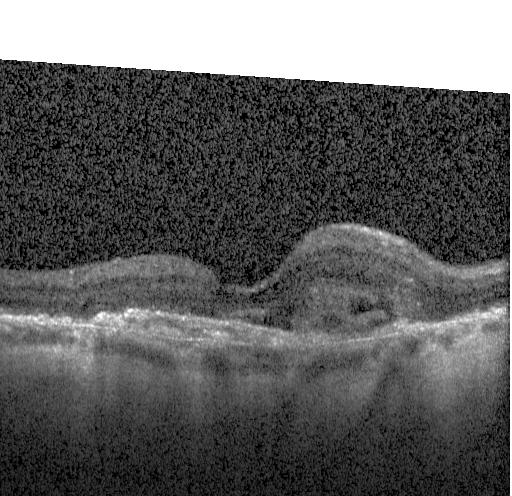 Heidelberg Spectralis; spectral-domain OCT; optical coherence tomography B-scan; through the macula
Macular OCT: choroidal neovascularization (CNV).